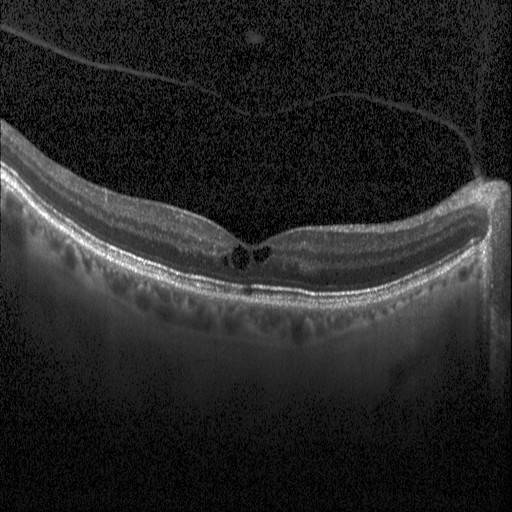 Retinal OCT B-scan.
Diagnosis: diabetic macular edema (DME).